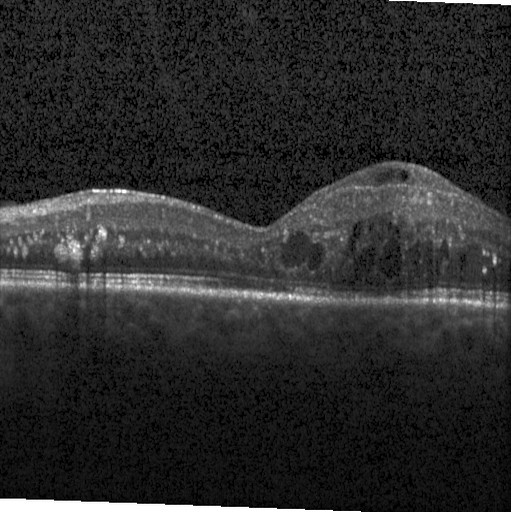

Spectral-domain optical coherence tomography · horizontal scan through the fovea · optical coherence tomography scan — Dx: diabetic macular edema (DME).